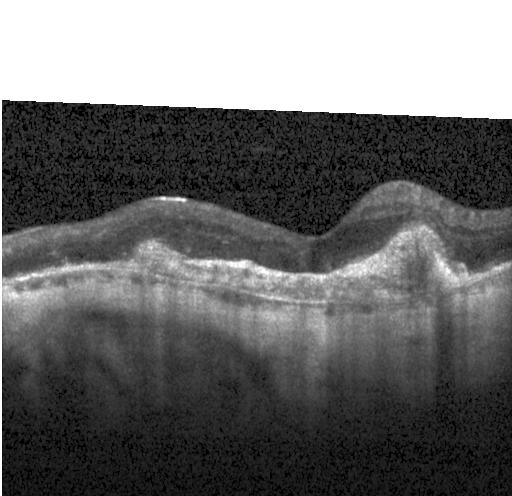

OCT line scan; spectral-domain optical coherence tomography. Finding: choroidal neovascularization (CNV).